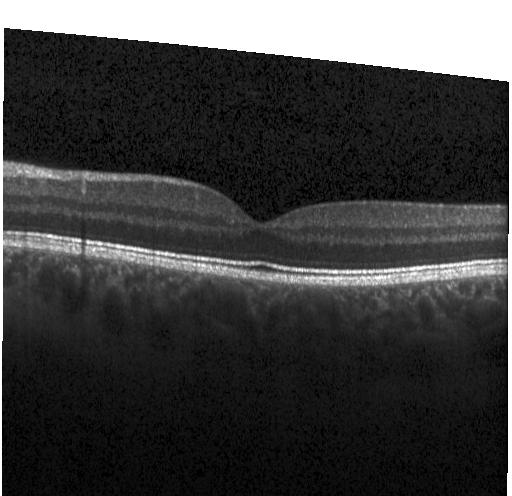

Centered on the fovea; Heidelberg Spectralis; retinal OCT cross-section; spectral-domain optical coherence tomography.
No CNV, no DME, and no drusen.